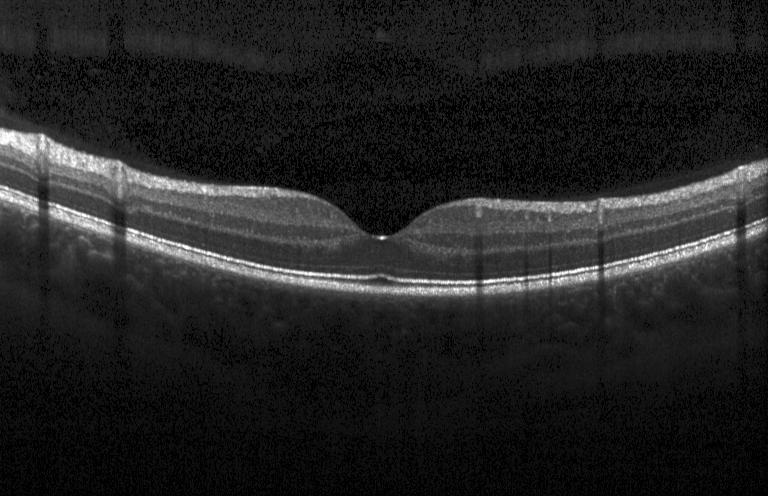 Retinal OCT B-scan. Spectral-domain OCT. Fovea-centered. Instrument: Heidelberg Spectralis — Diagnosis: no choroidal neovascularization, no diabetic macular edema, and no drusen.